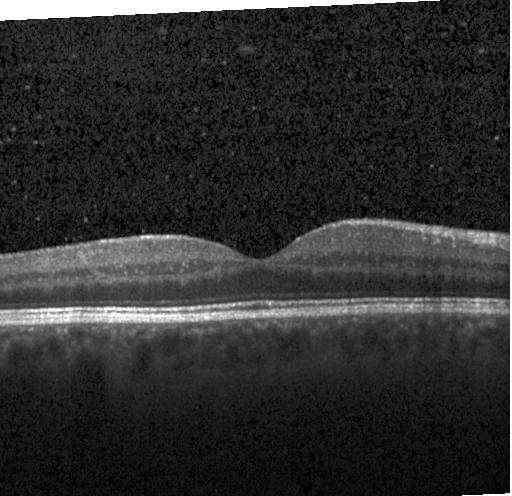
Assessment: no evidence of choroidal neovascularization, diabetic macular edema, or drusen.